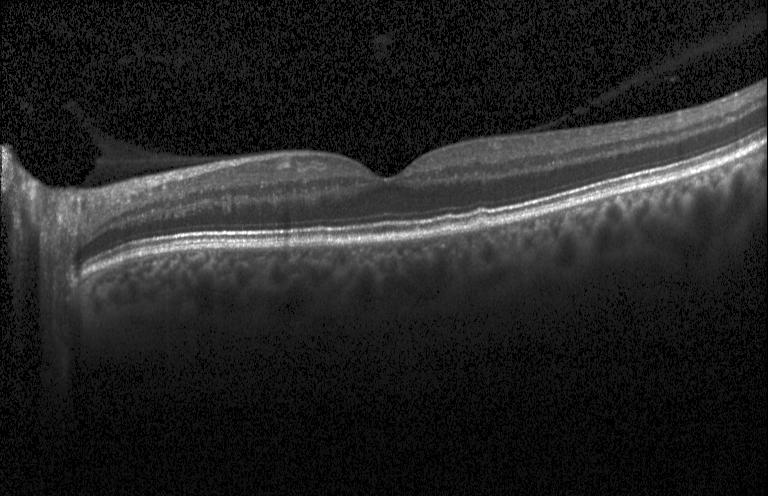
Retinal OCT cross-section showing no choroidal neovascularization, diabetic macular edema, or drusen.